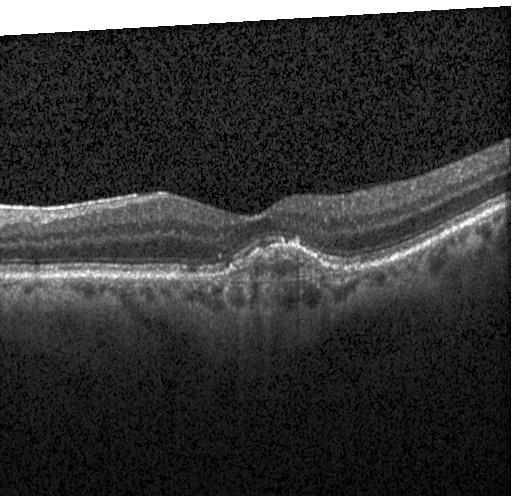 Assessment: choroidal neovascularization (CNV).